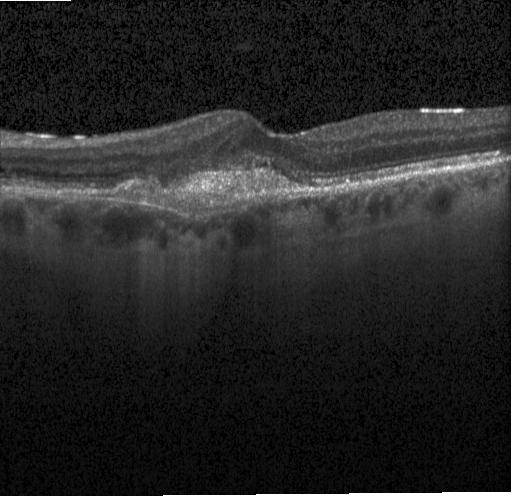 Retinal OCT cross-section showing a choroidal neovascular membrane.